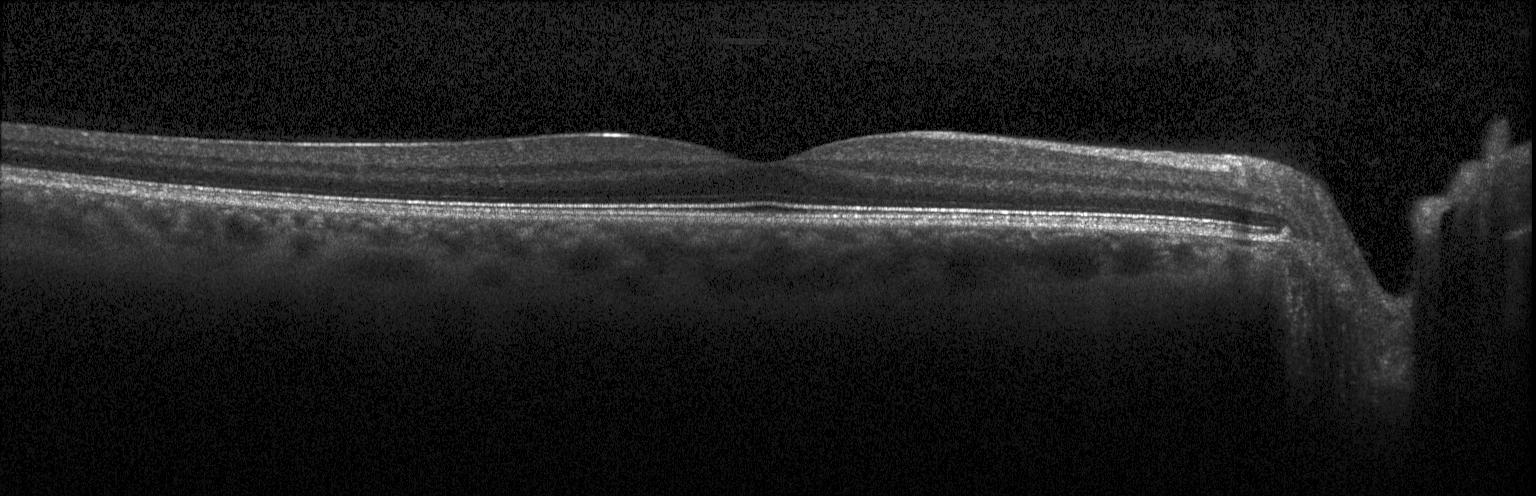
Heidelberg Spectralis OCT system; optical coherence tomography B-scan; through the macula; SD-OCT
Impression: no CNV, no DME, and no drusen.